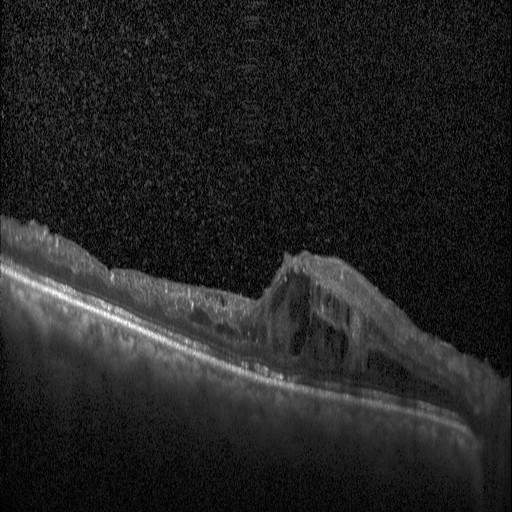
Spectral-domain optical coherence tomography · macular scan · OCT line scan
The scan shows diabetic macular edema.